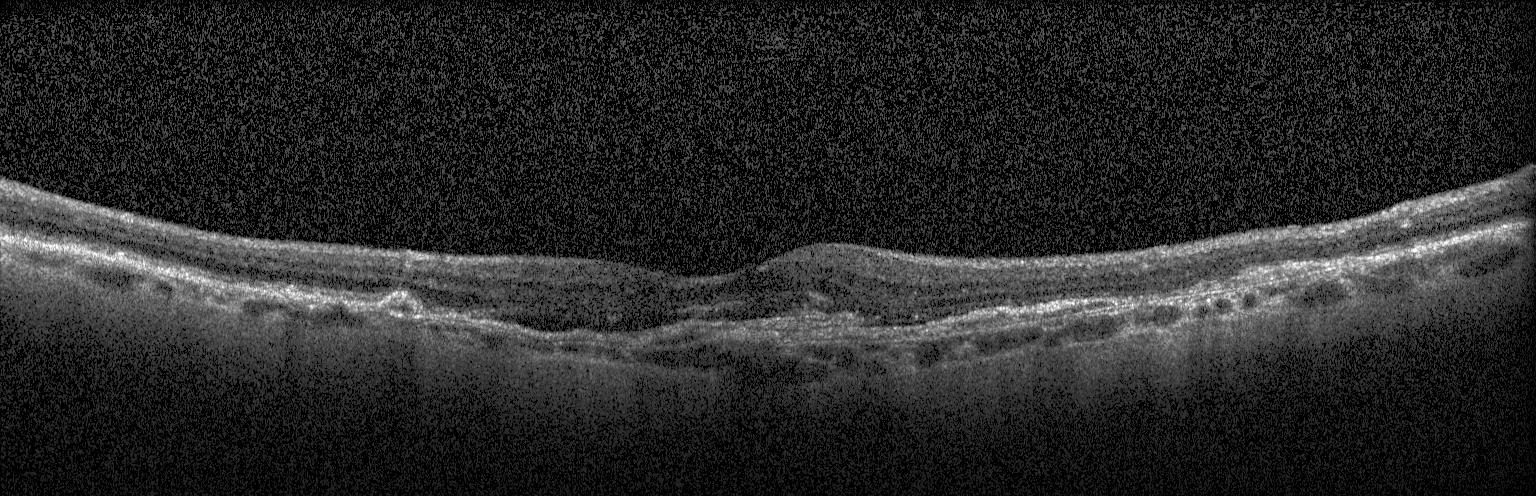
Macular OCT: a choroidal neovascular membrane.